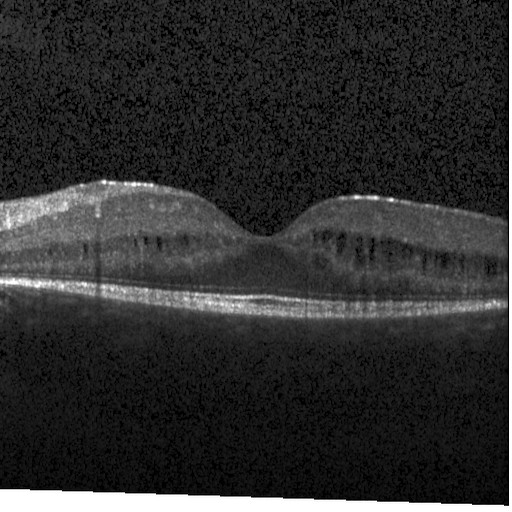
Optical coherence tomography B-scan. Diagnosis: diabetic macular edema.